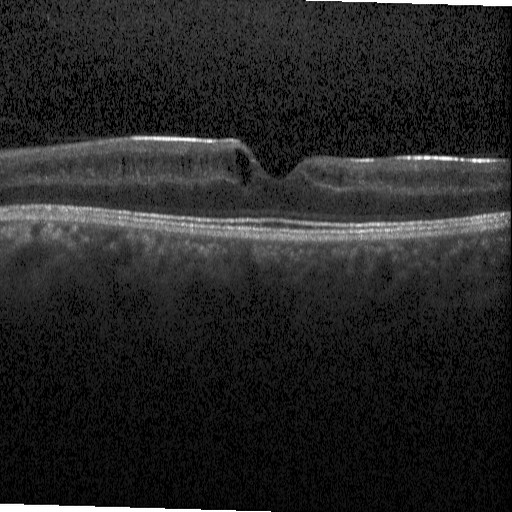 Heidelberg Spectralis; retinal OCT B-scan — This B-scan demonstrates diabetic macular edema (DME).